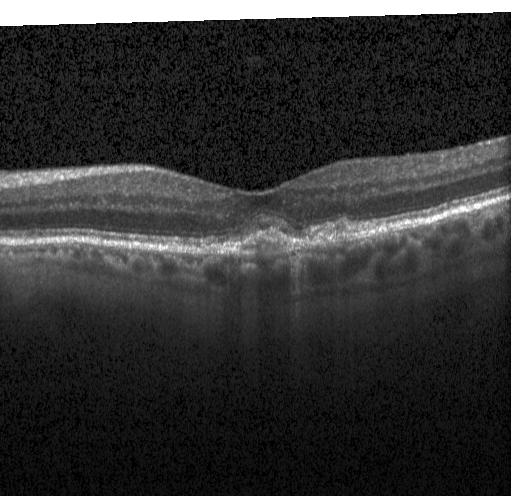 OCT B-scan, Heidelberg Spectralis, SD-OCT, through the macula.
Finding: a choroidal neovascular membrane.